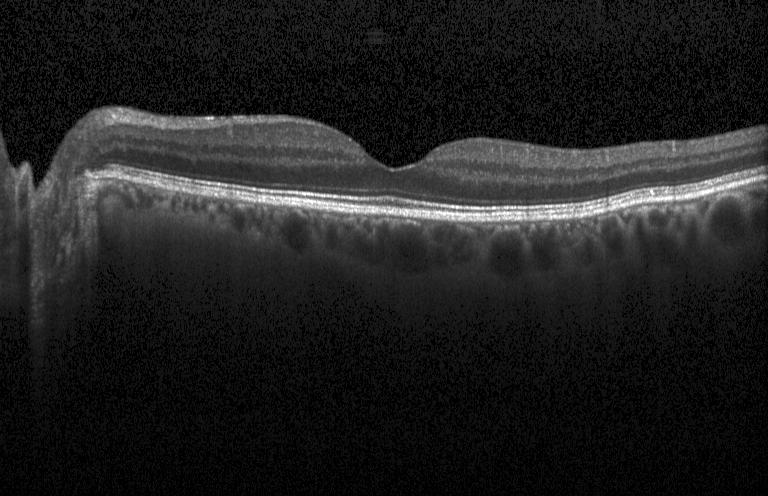

Retinal OCT cross-section. The scan shows no evidence of CNV, DME, or drusen.